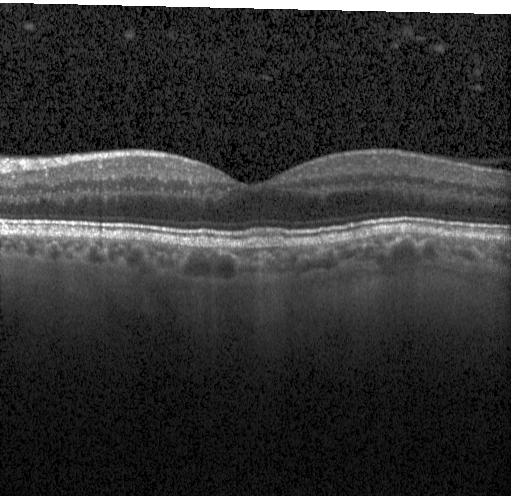 Fovea-centered · acquired on a Heidelberg Spectralis · retinal OCT B-scan
OCT finding: no evidence of choroidal neovascularization, diabetic macular edema, or drusen.